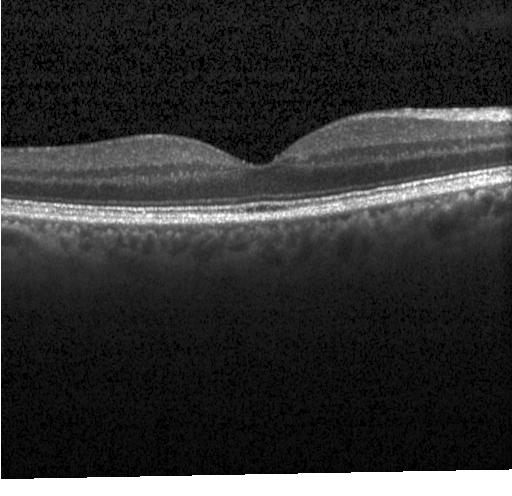

Optical coherence tomography B-scan — Diagnosis: neither CNV, DME, nor drusen.